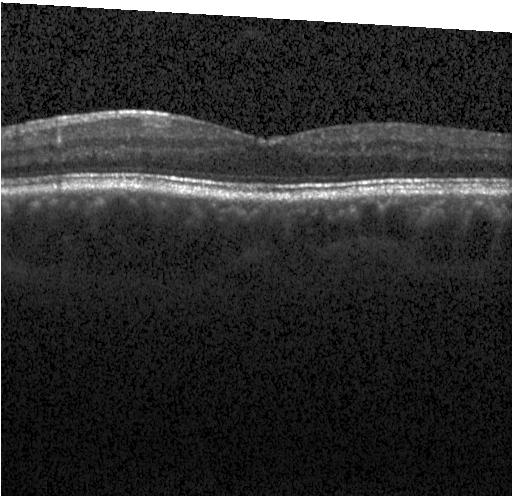
Impression: no evidence of CNV, DME, or drusen.